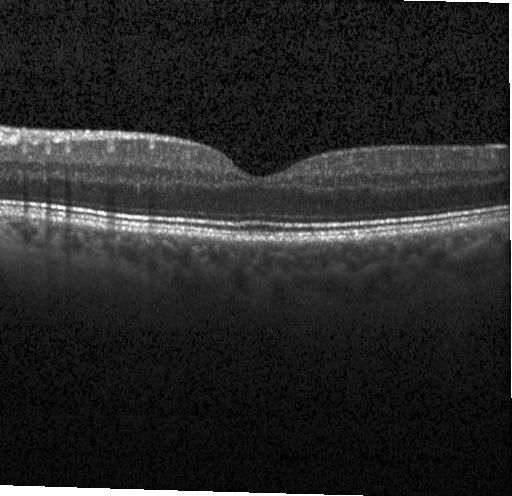 Instrument: Heidelberg Spectralis · OCT B-scan · spectral-domain OCT · fovea-centered.
Macular OCT: no CNV, DME, or drusen.